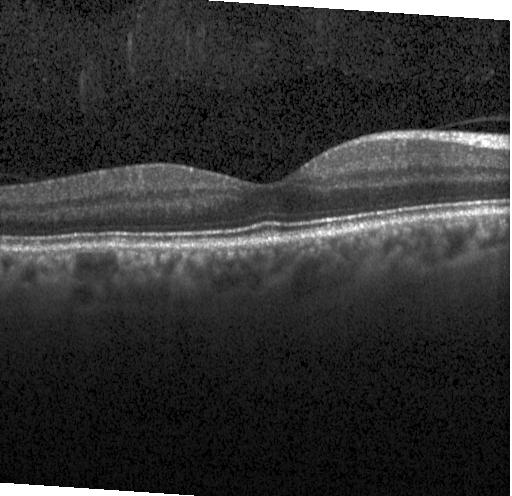

Optical coherence tomography B-scan · macular scan
Diagnosis: no choroidal neovascularization, diabetic macular edema, or drusen.